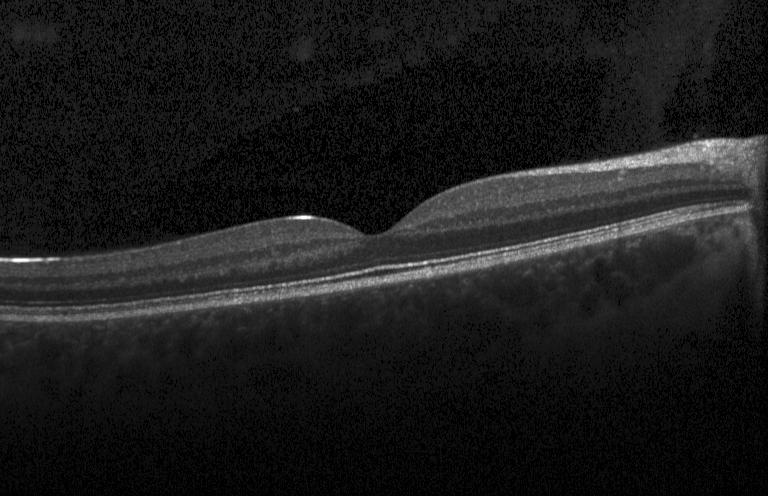 Macular scan; acquired on a Heidelberg Spectralis; OCT line scan.
Impression: no evidence of choroidal neovascularization, diabetic macular edema, or drusen.